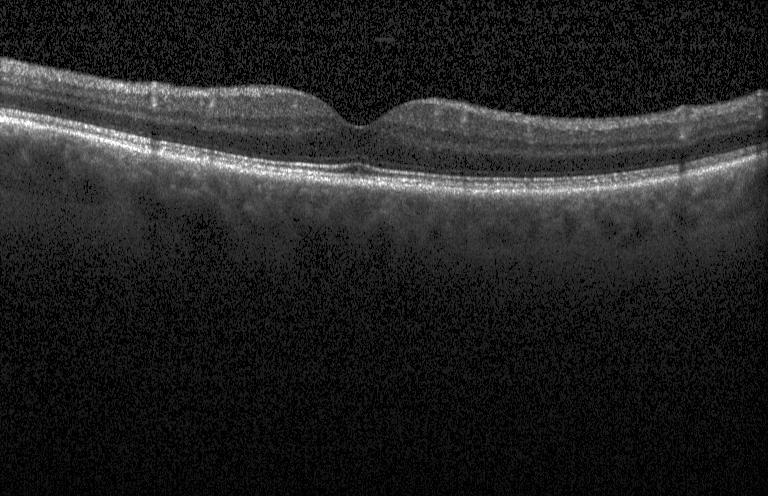
Assessment: no choroidal neovascularization, diabetic macular edema, or drusen.